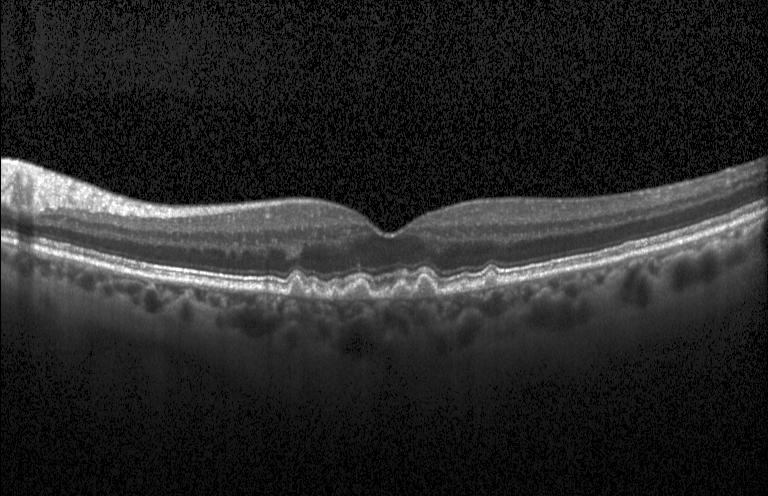
Diagnosis: multiple drusen.